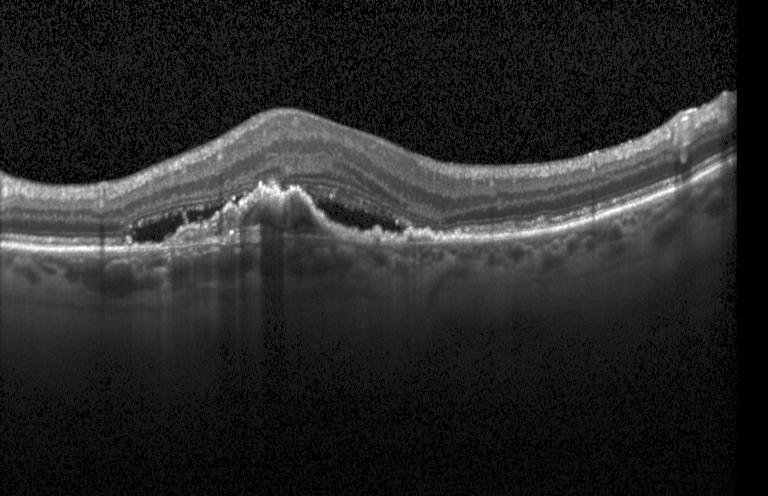
Retinal OCT cross-section. Assessment: a choroidal neovascular membrane.